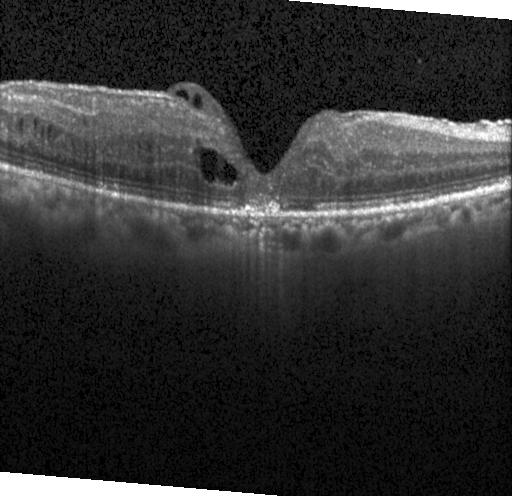

Retinal OCT B-scan; fovea-centered — Finding: DME.